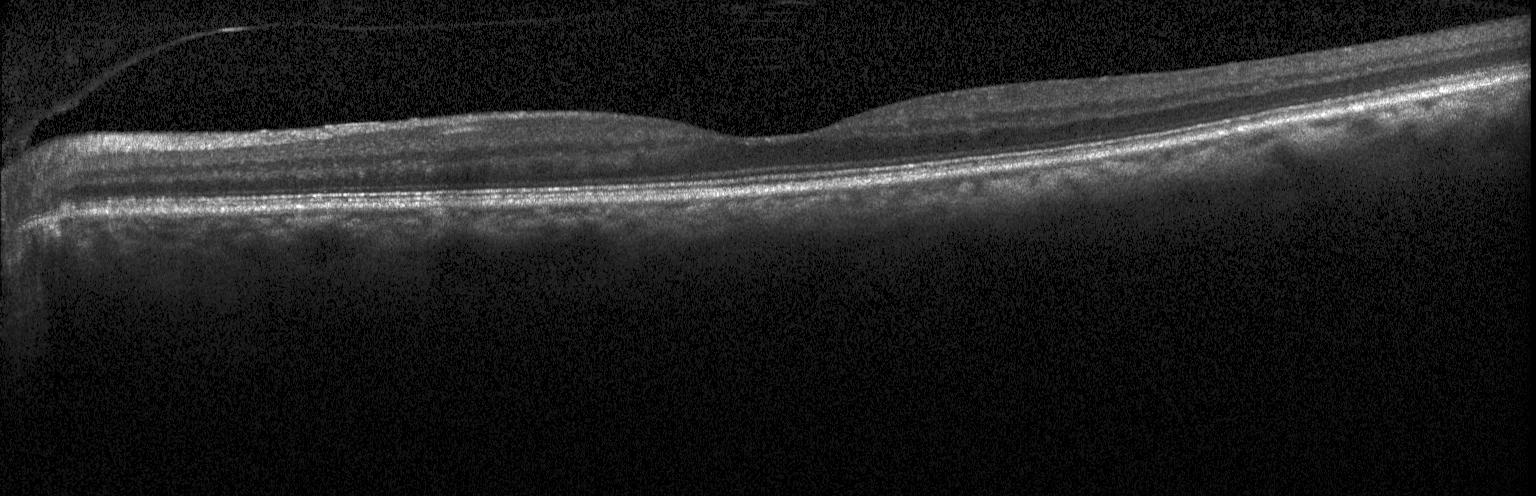
Macular OCT demonstrating no choroidal neovascularization, no diabetic macular edema, and no drusen.